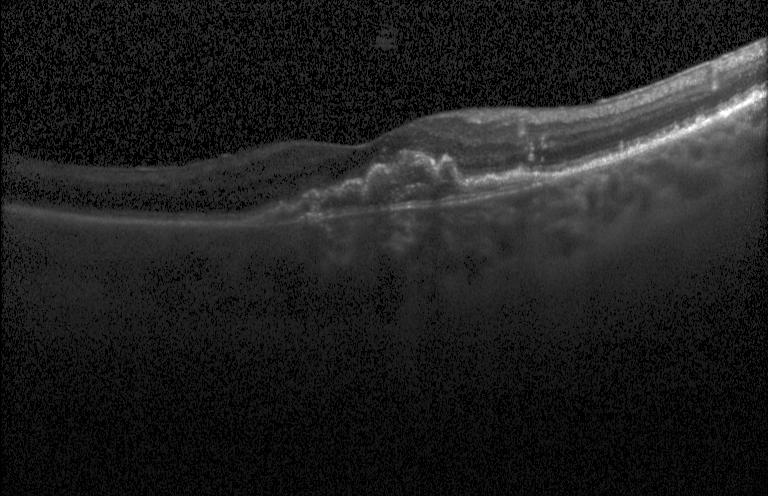

OCT line scan — Dx: CNV.